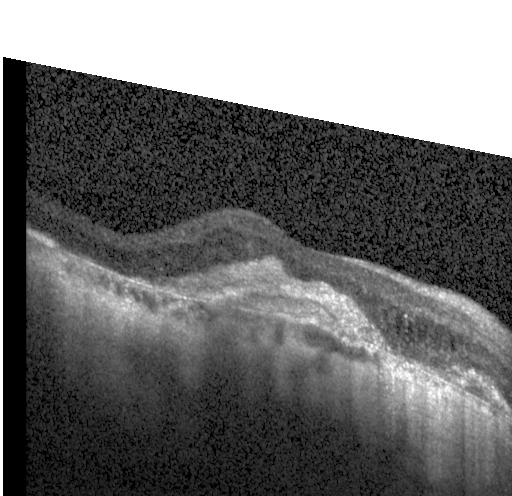
Impression: CNV.